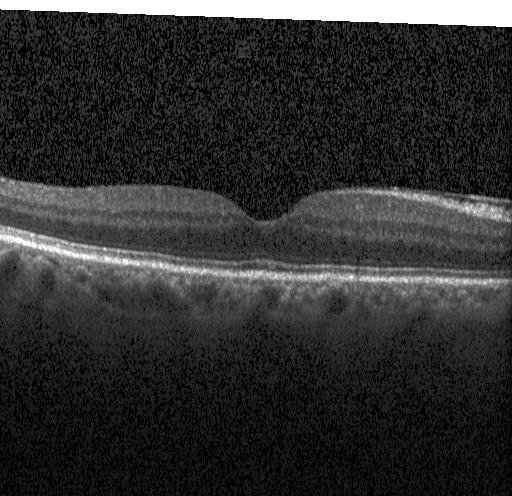

Spectral-domain OCT; instrument: Heidelberg Spectralis; centered on the fovea; retinal OCT cross-section.
Diagnosis: no CNV, DME, or drusen.